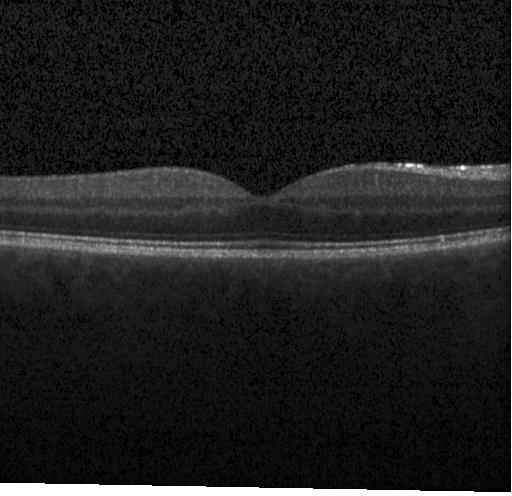
Assessment: no evidence of choroidal neovascularization, diabetic macular edema, or drusen.